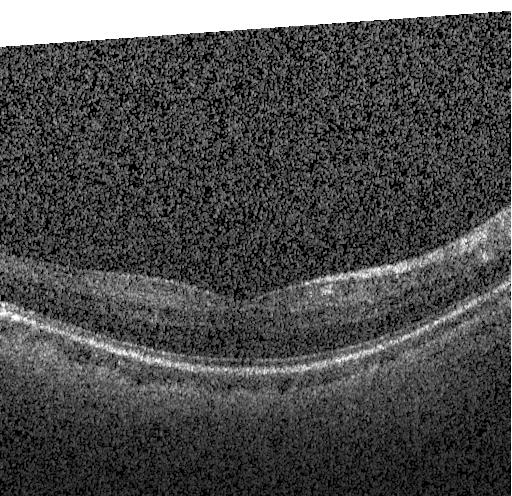
Optical coherence tomography B-scan · Heidelberg Spectralis · SD-OCT — Diagnosis: no evidence of CNV, DME, or drusen.